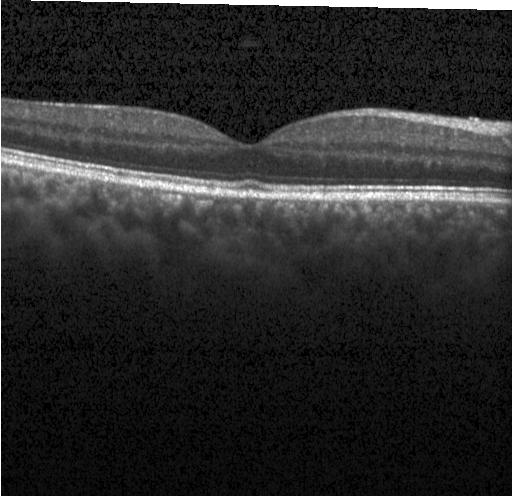 Retinal OCT B-scan, Heidelberg Spectralis.
OCT finding: no choroidal neovascularization, diabetic macular edema, or drusen.